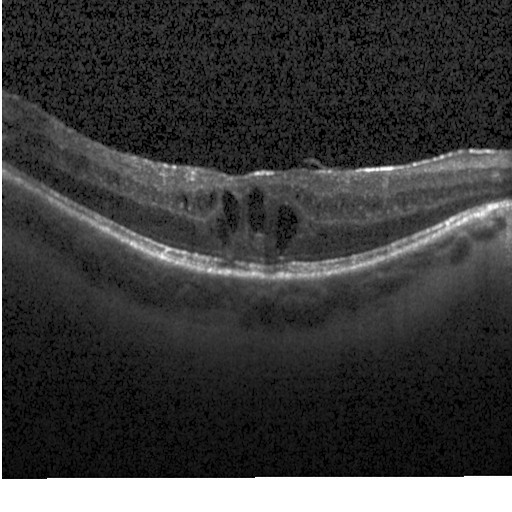

Spectral-domain optical coherence tomography · instrument: Heidelberg Spectralis · optical coherence tomography scan · through the macula. OCT finding: diabetic macular edema (DME).